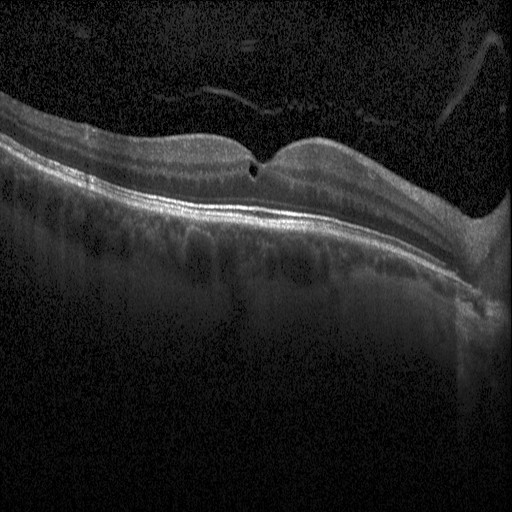

Diagnosis: diabetic macular edema (DME).